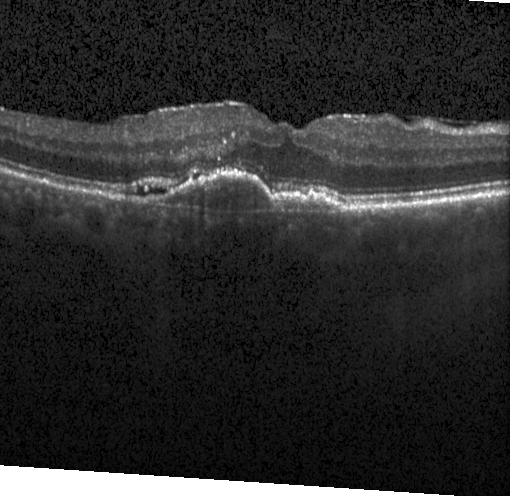 Choroidal neovascularization (CNV).